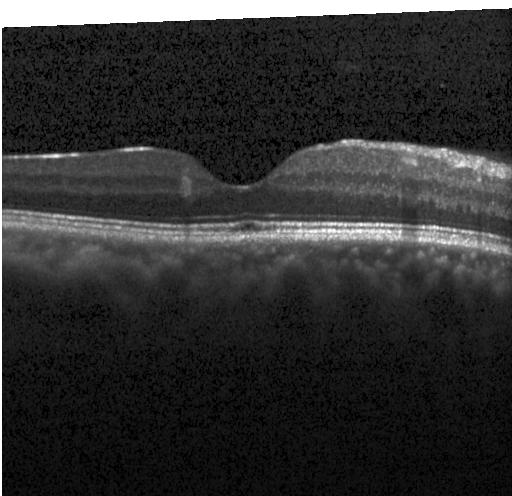

Instrument: Heidelberg Spectralis. Through the macula. Retinal OCT cross-section. Spectral-domain OCT
Diagnosis: no CNV, DME, or drusen.